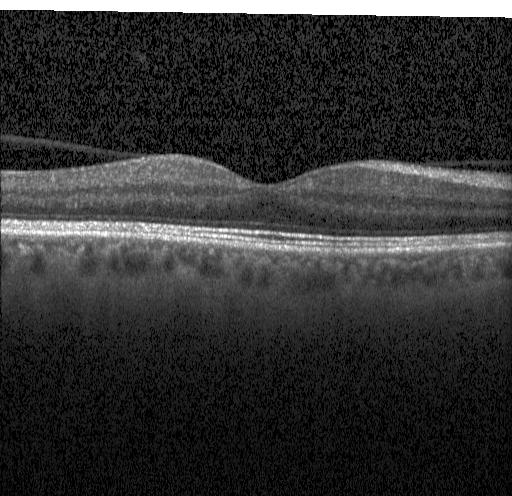
Spectral-domain OCT B-scan: no evidence of choroidal neovascularization, diabetic macular edema, or drusen.